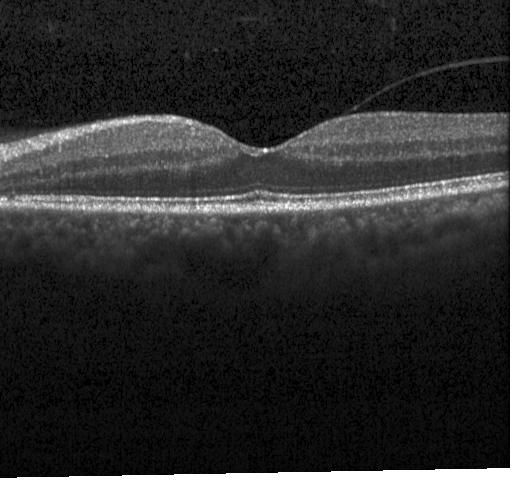
Retinal OCT B-scan. Fovea-centered — Assessment: no CNV, DME, or drusen.